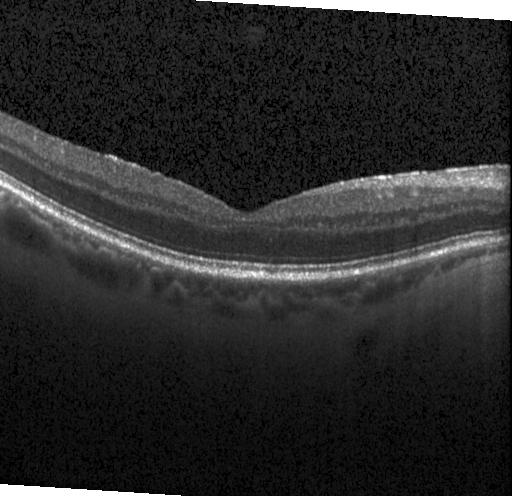
Spectral-domain OCT B-scan: neither choroidal neovascularization, diabetic macular edema, nor drusen.